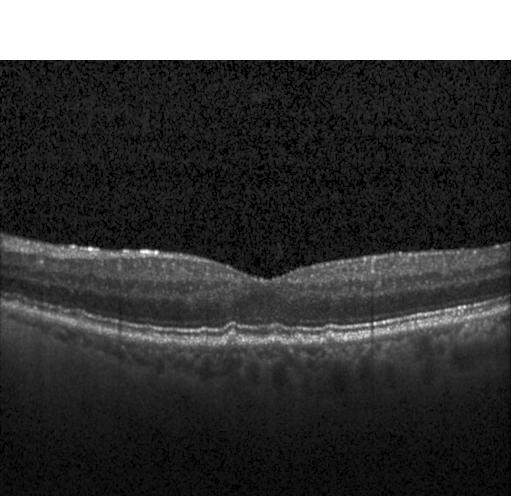

SD-OCT · Heidelberg Spectralis OCT system · optical coherence tomography scan · fovea-centered — Multiple drusen.